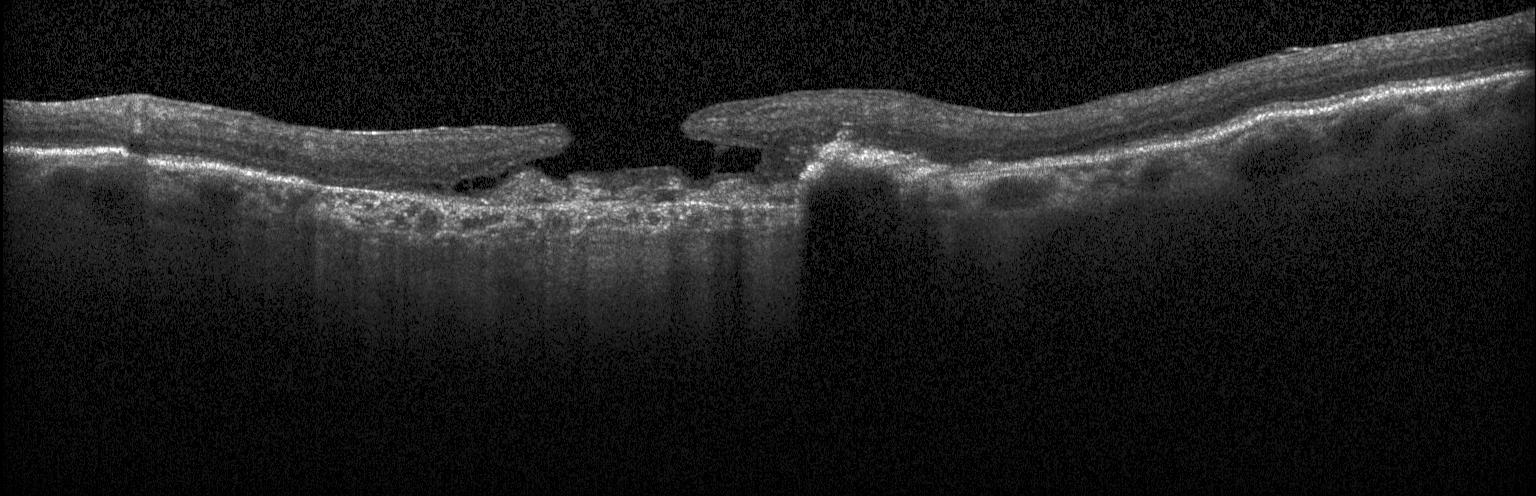 Impression: choroidal neovascularization (CNV).